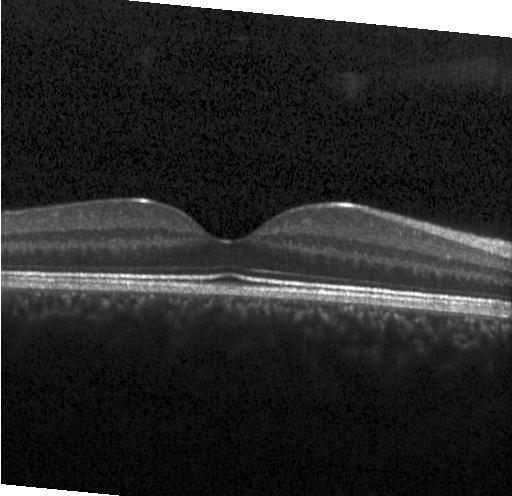

Retinal OCT cross-section, macular scan — Diagnosis: no choroidal neovascularization, no diabetic macular edema, and no drusen.